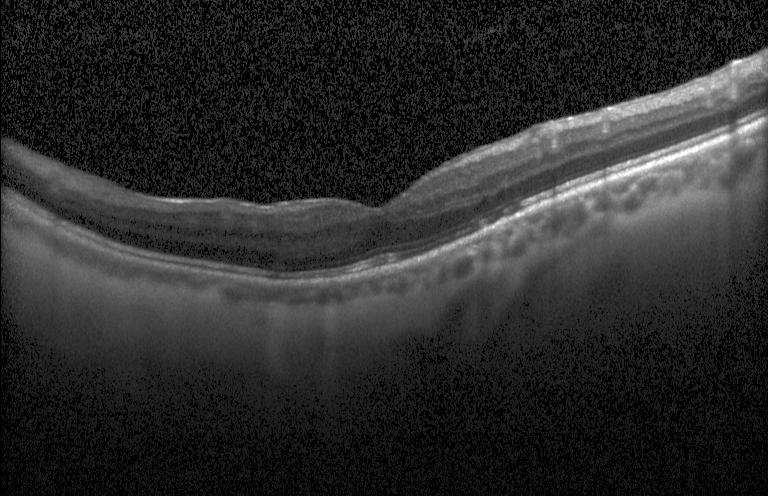 Heidelberg Spectralis. Horizontal scan through the fovea. Optical coherence tomography scan. Spectral-domain OCT
Impression: no choroidal neovascularization, diabetic macular edema, or drusen.